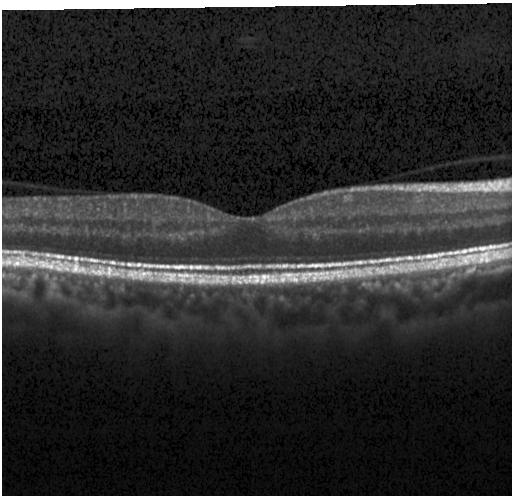

Macular OCT: no choroidal neovascularization, diabetic macular edema, or drusen.